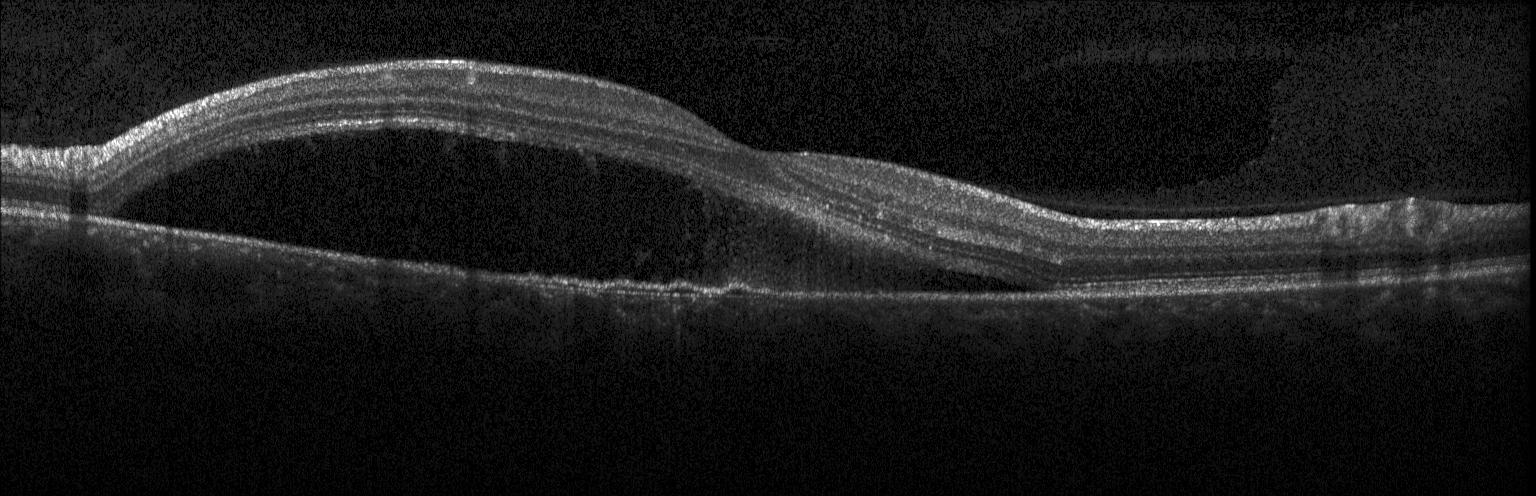 Optical coherence tomography scan
Macular OCT: choroidal neovascularization.